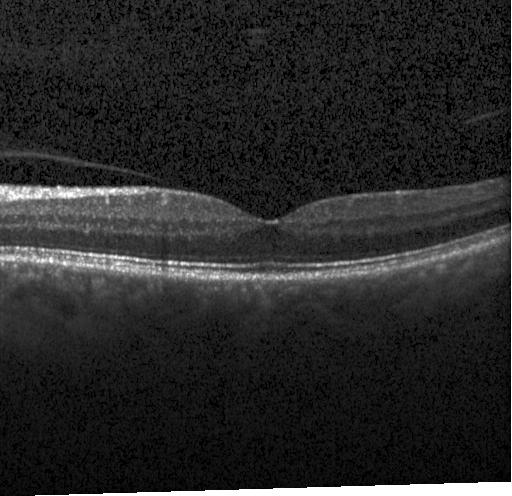

Diagnosis: neither CNV, DME, nor drusen.